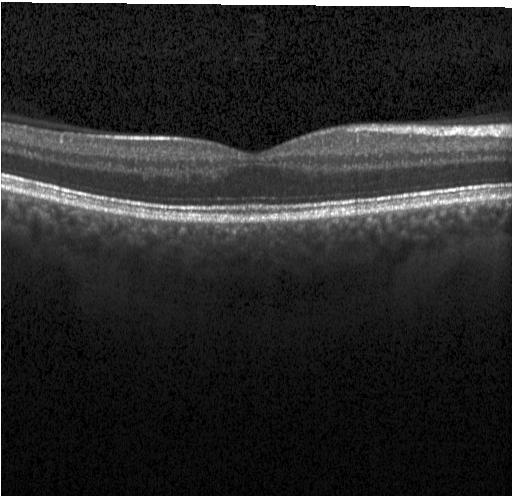

Spectral-domain OCT B-scan: no choroidal neovascularization, diabetic macular edema, or drusen.